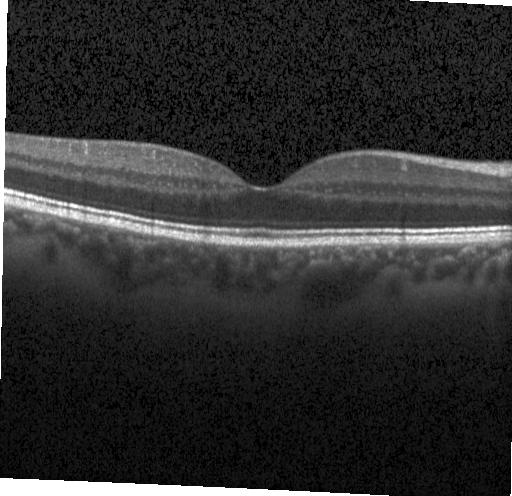
Optical coherence tomography scan; instrument: Heidelberg Spectralis. Dx: no CNV, no DME, and no drusen.